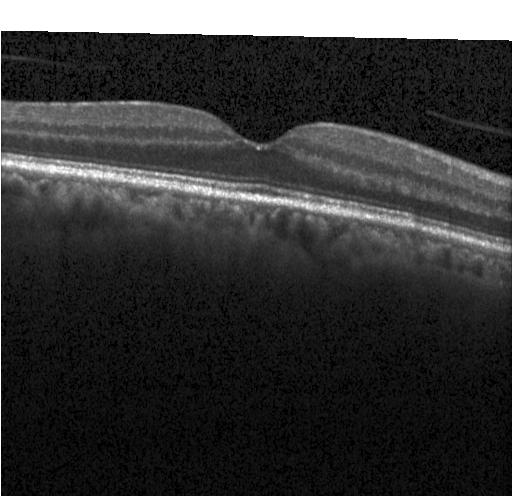 Impression: no CNV, no DME, and no drusen.